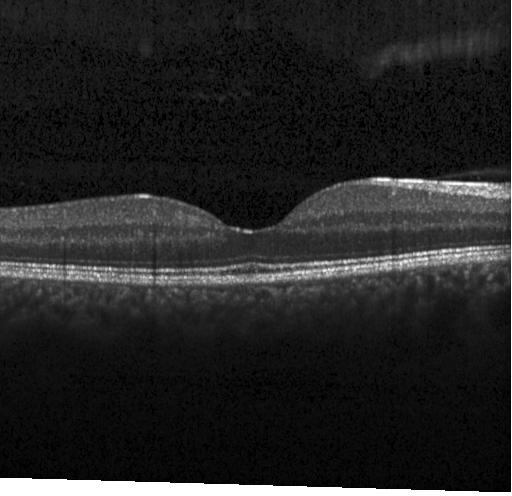

Macular OCT: no evidence of choroidal neovascularization, diabetic macular edema, or drusen.